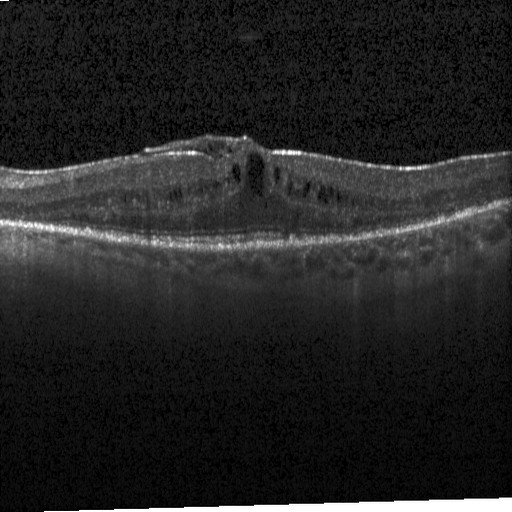

Through the macula, optical coherence tomography B-scan, Heidelberg Spectralis. Diabetic macular edema (DME).